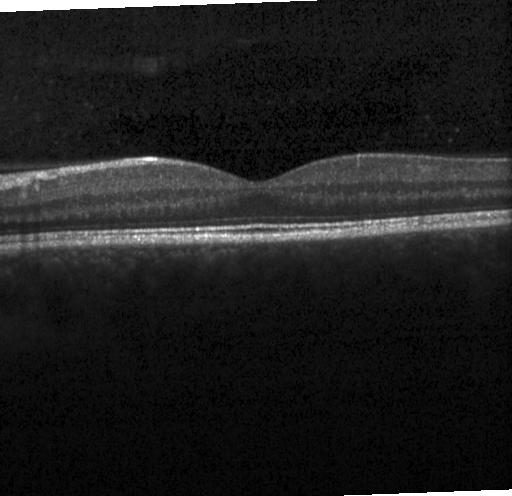 The scan shows no CNV, no DME, and no drusen.